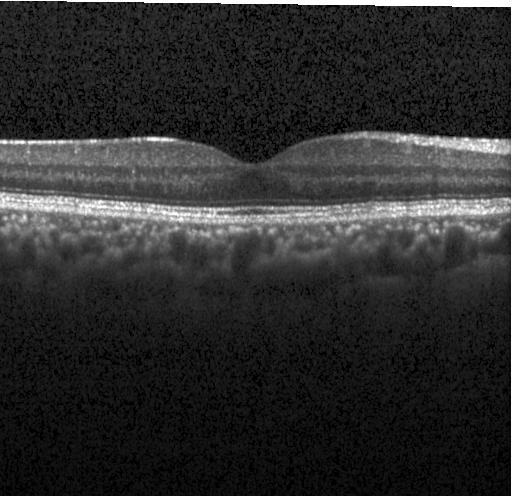 Finding: no CNV, no DME, and no drusen.